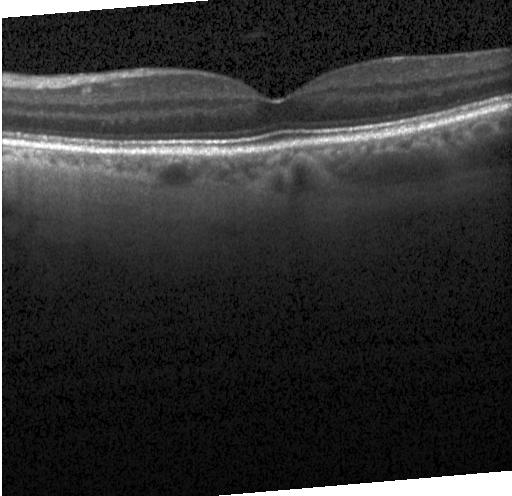
Macular scan · SD-OCT · instrument: Heidelberg Spectralis · optical coherence tomography scan
Finding: neither CNV, DME, nor drusen.